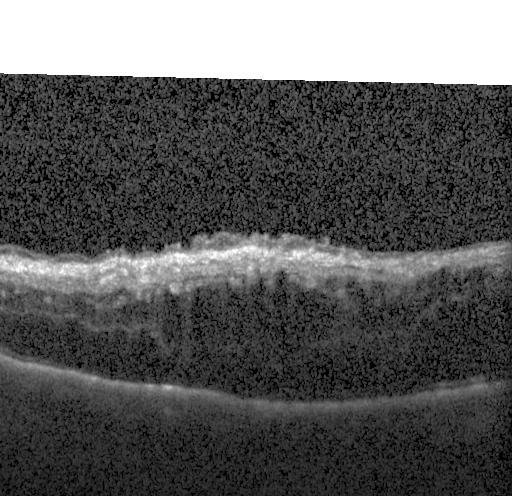

Heidelberg Spectralis OCT system. Fovea-centered. OCT line scan.
This B-scan demonstrates diabetic macular edema.